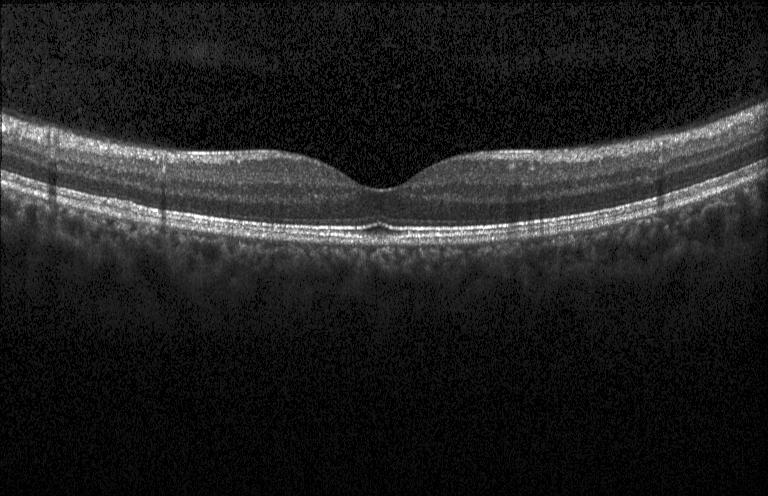

Finding: no evidence of choroidal neovascularization, diabetic macular edema, or drusen.